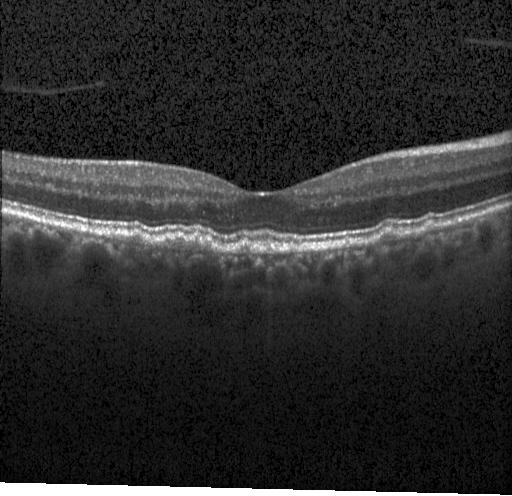 Retinal OCT cross-section
The scan shows drusen.